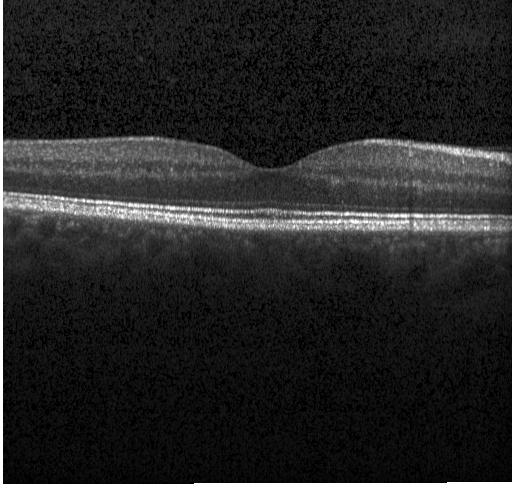 Macular OCT demonstrating no evidence of choroidal neovascularization, diabetic macular edema, or drusen.